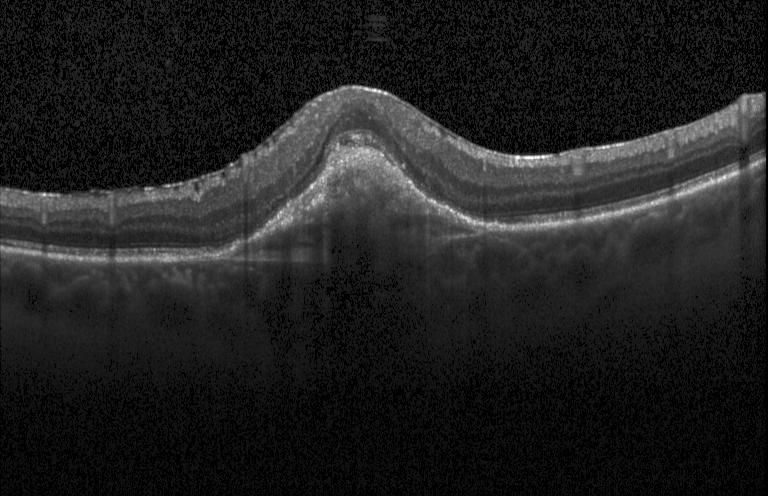 OCT finding: a choroidal neovascular membrane.